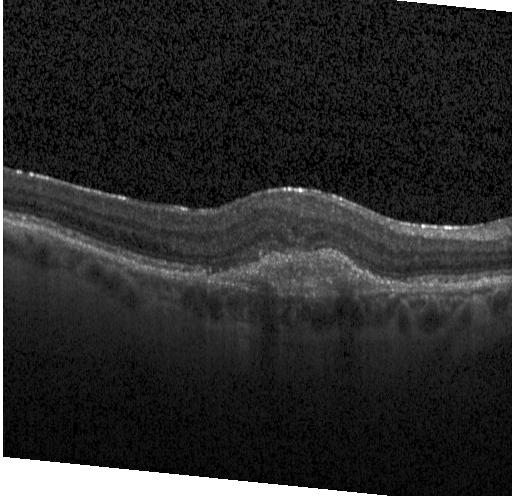

Macular OCT: a choroidal neovascular membrane.